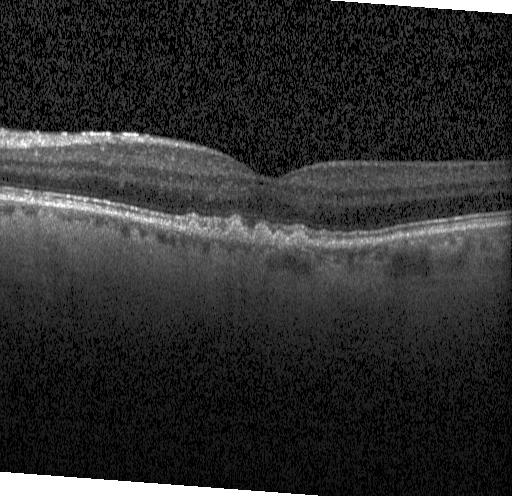 Retinal OCT B-scan
The scan shows multiple drusen.